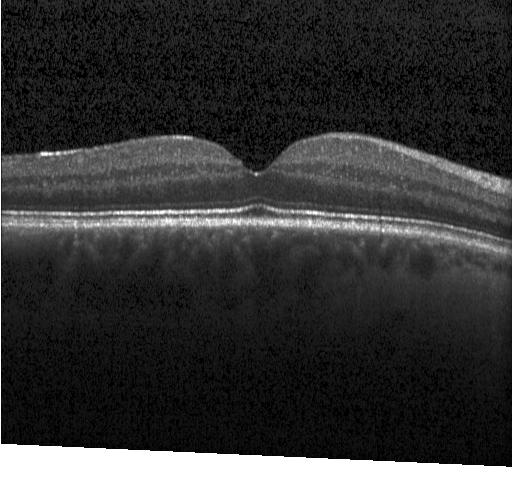

OCT scan showing no evidence of choroidal neovascularization, diabetic macular edema, or drusen.